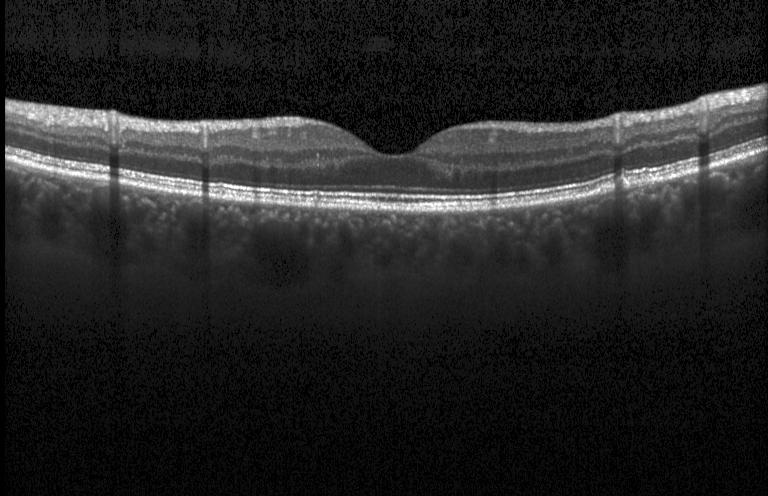 Acquired on a Heidelberg Spectralis · optical coherence tomography scan — Macular OCT: no choroidal neovascularization, diabetic macular edema, or drusen.